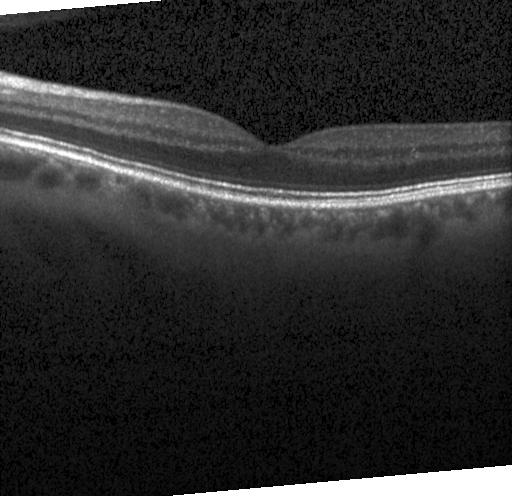 Assessment: no choroidal neovascularization, diabetic macular edema, or drusen.